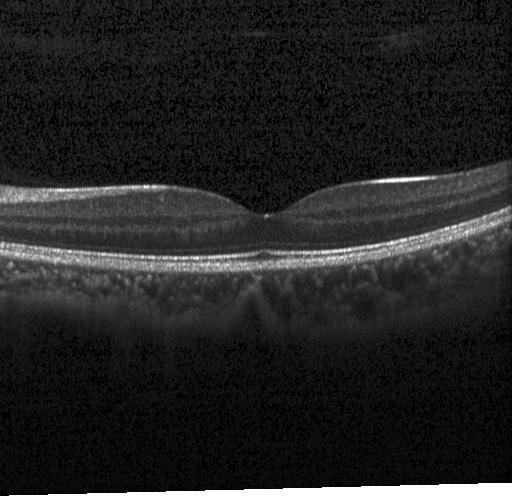

OCT B-scan, through the macula, instrument: Heidelberg Spectralis.
This B-scan demonstrates neither choroidal neovascularization, diabetic macular edema, nor drusen.